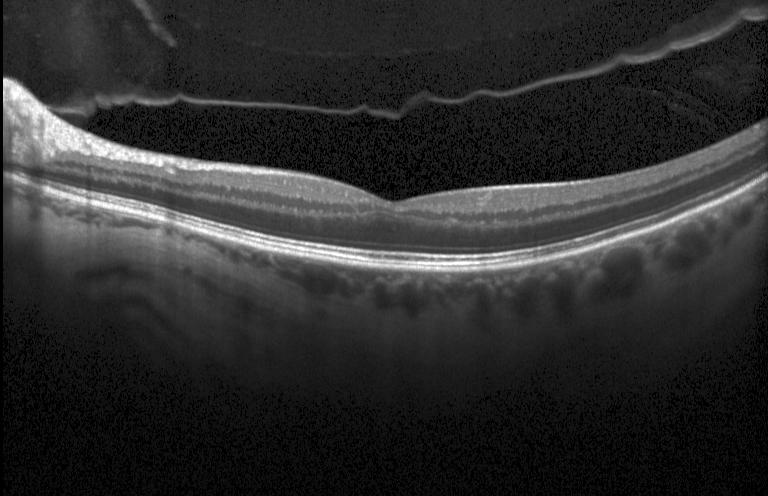
Heidelberg Spectralis, through the macula, retinal OCT B-scan, spectral-domain OCT. Finding: no CNV, no DME, and no drusen.